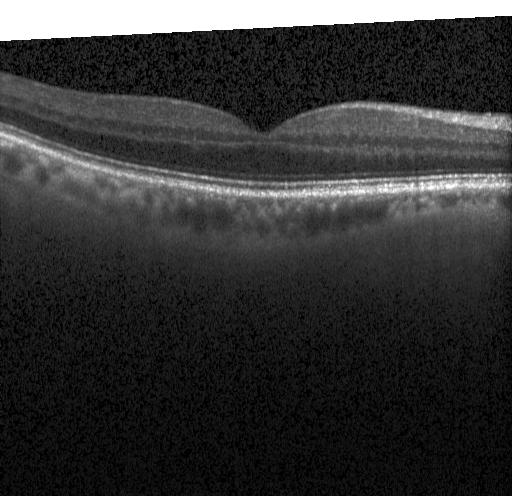

Spectral-domain optical coherence tomography, retinal OCT cross-section, Heidelberg Spectralis, macular scan.
Finding: no CNV, DME, or drusen.